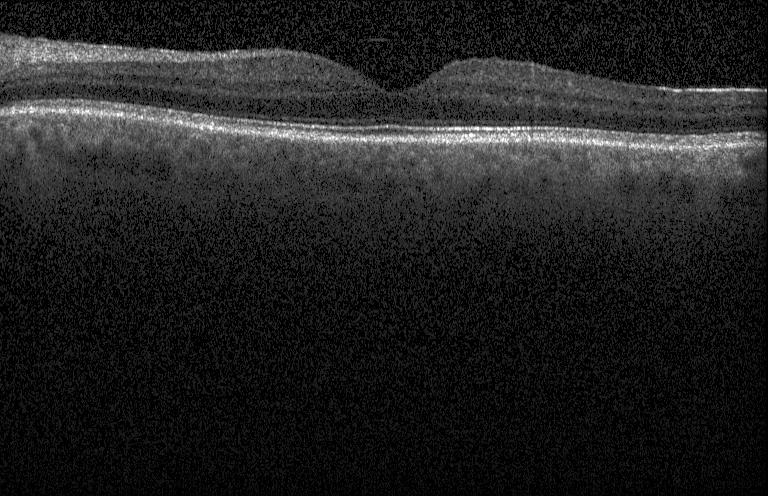

OCT scan showing no CNV, DME, or drusen.